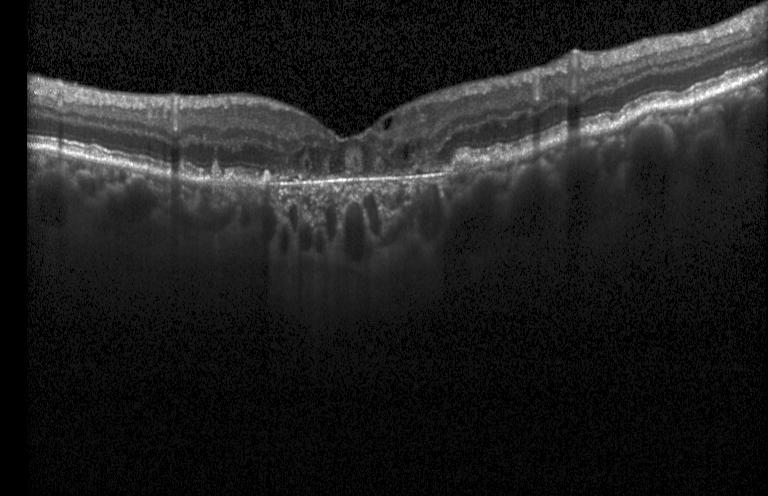
Assessment: a choroidal neovascular membrane.